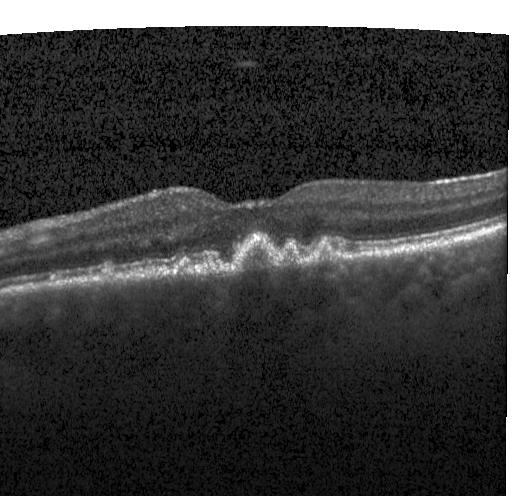
Instrument: Heidelberg Spectralis · spectral-domain OCT · horizontal scan through the fovea · retinal OCT cross-section — Finding: sub-RPE drusenoid deposits.